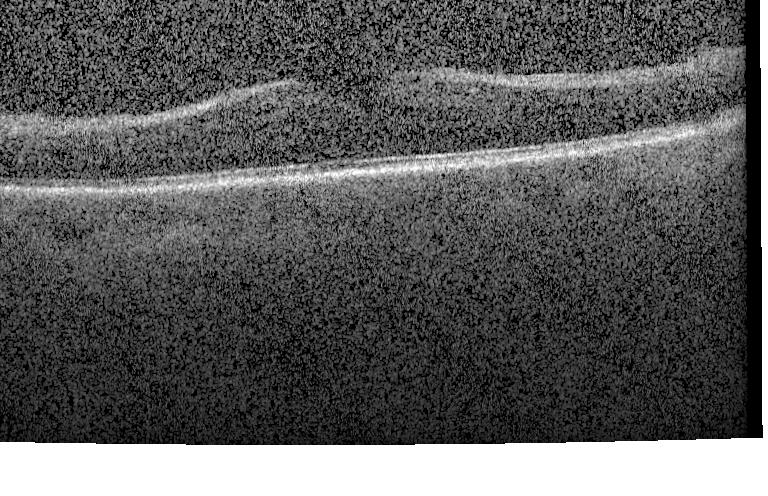 OCT line scan; through the macula; instrument: Heidelberg Spectralis; spectral-domain OCT — Diagnosis: no evidence of choroidal neovascularization, diabetic macular edema, or drusen.